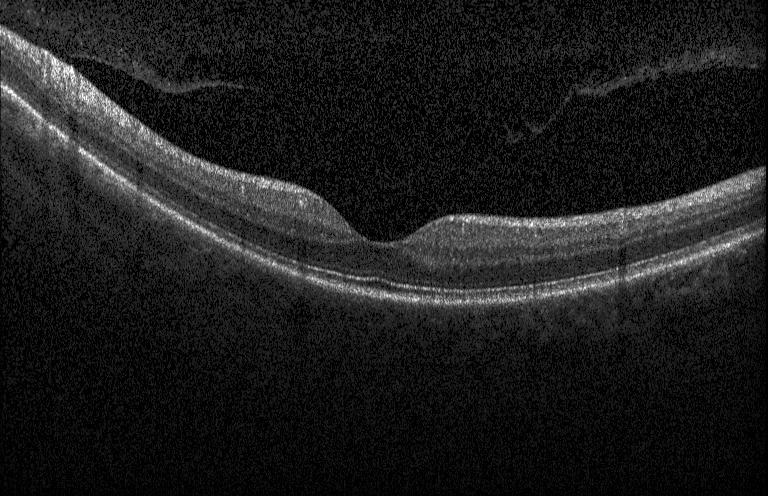 Heidelberg Spectralis, retinal OCT cross-section, macular scan, SD-OCT
Dx: neither choroidal neovascularization, diabetic macular edema, nor drusen.